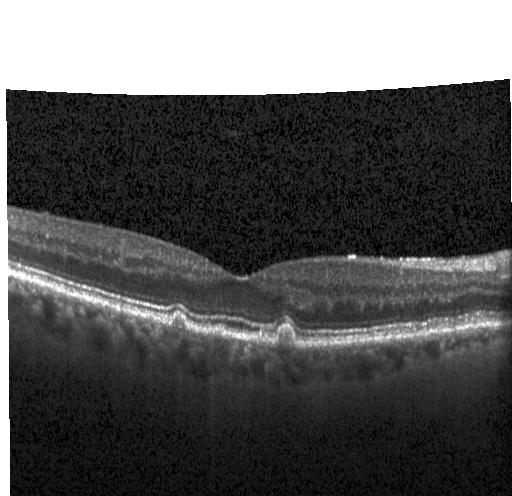
Macular OCT: multiple drusen.